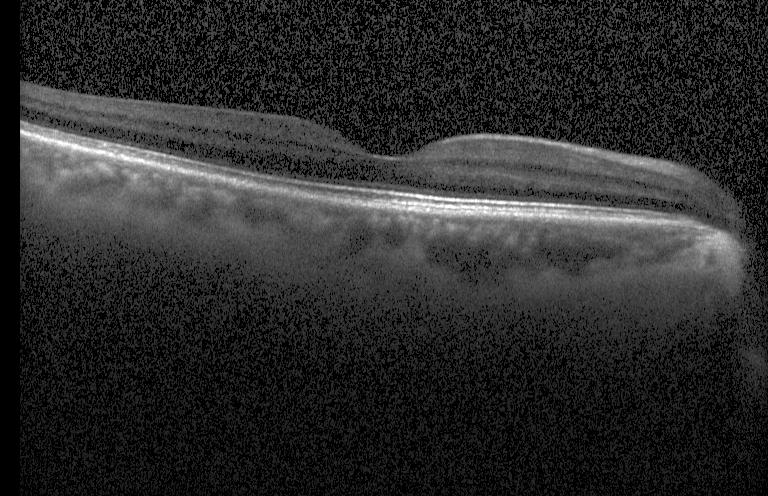 Finding: no evidence of CNV, DME, or drusen.